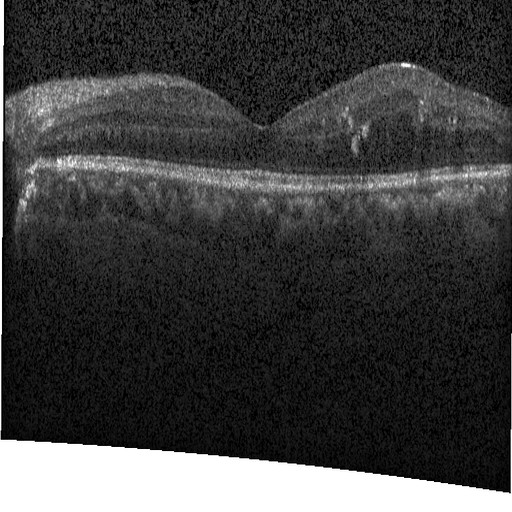
Retinal OCT cross-section. SD-OCT — Diabetic macular edema.